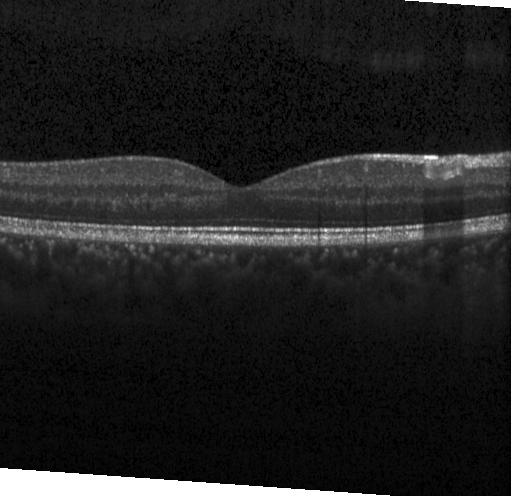

Heidelberg Spectralis OCT system; OCT B-scan. Finding: no CNV, no DME, and no drusen.